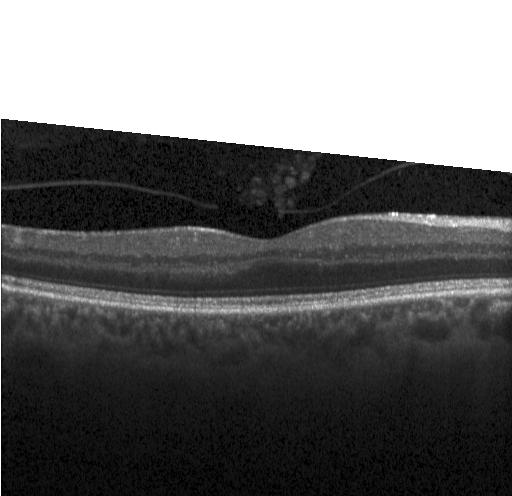 Horizontal scan through the fovea, Heidelberg Spectralis OCT system, OCT line scan, spectral-domain optical coherence tomography
Assessment: no CNV, no DME, and no drusen.